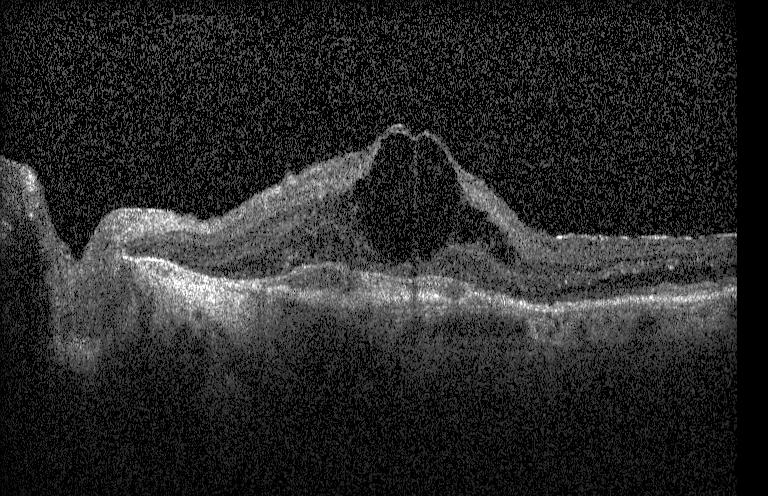

Spectral-domain optical coherence tomography · Heidelberg Spectralis · optical coherence tomography B-scan · fovea-centered — OCT finding: choroidal neovascularization (CNV).